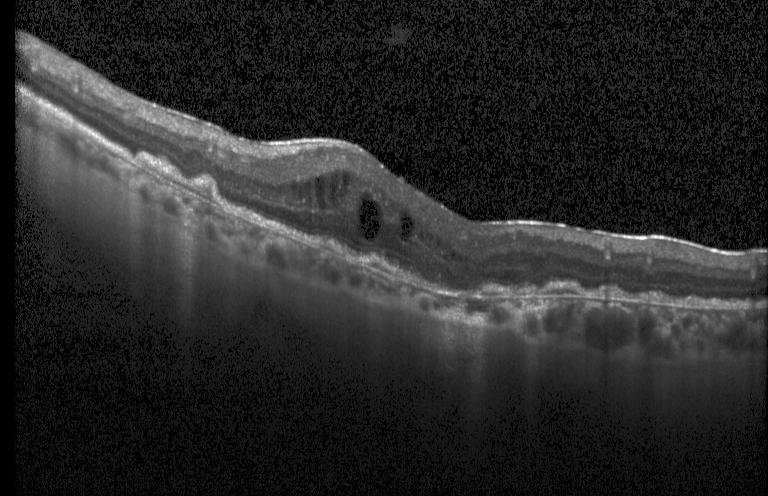 OCT line scan
Finding: choroidal neovascularization.